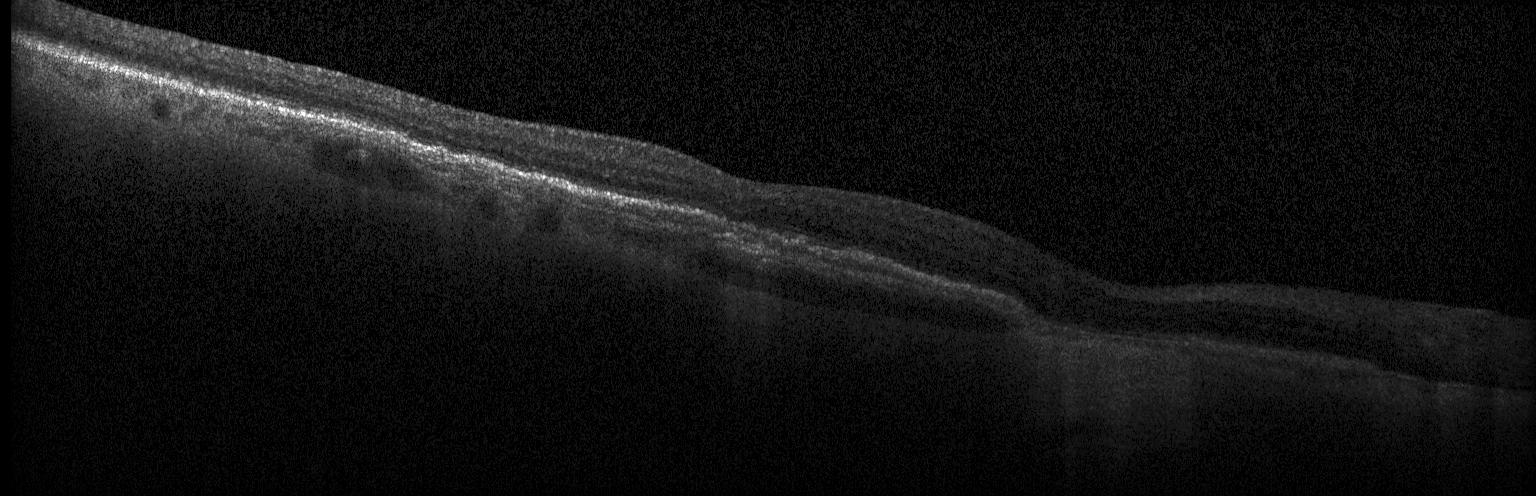

Optical coherence tomography B-scan; horizontal scan through the fovea; acquired on a Heidelberg Spectralis; SD-OCT. Finding: a choroidal neovascular membrane.